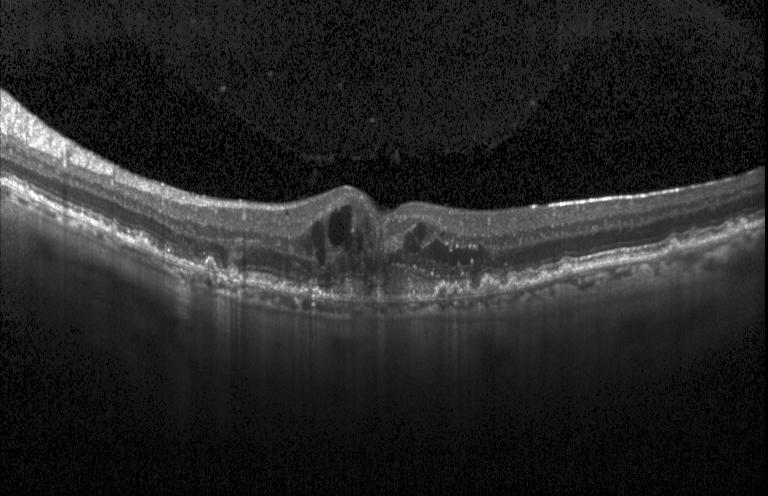

Diagnosis: choroidal neovascularization (CNV).